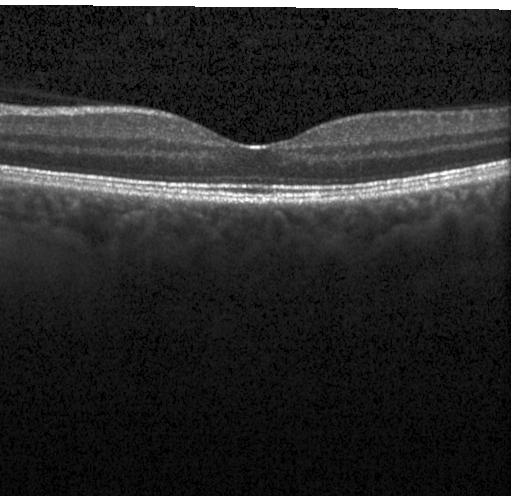
Retinal OCT cross-section
The scan shows no CNV, DME, or drusen.